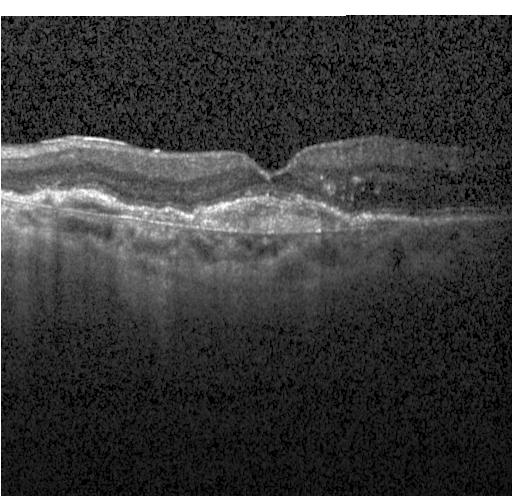
Heidelberg Spectralis, OCT line scan. A choroidal neovascular membrane.